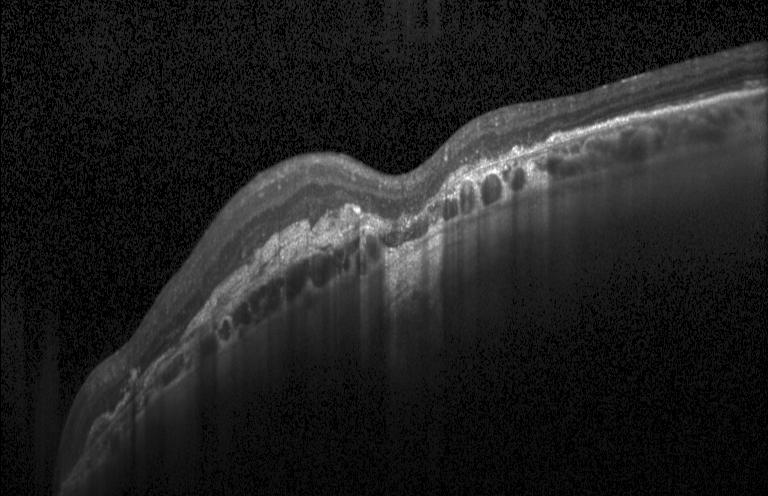 Acquired on a Heidelberg Spectralis · OCT B-scan
Choroidal neovascularization.